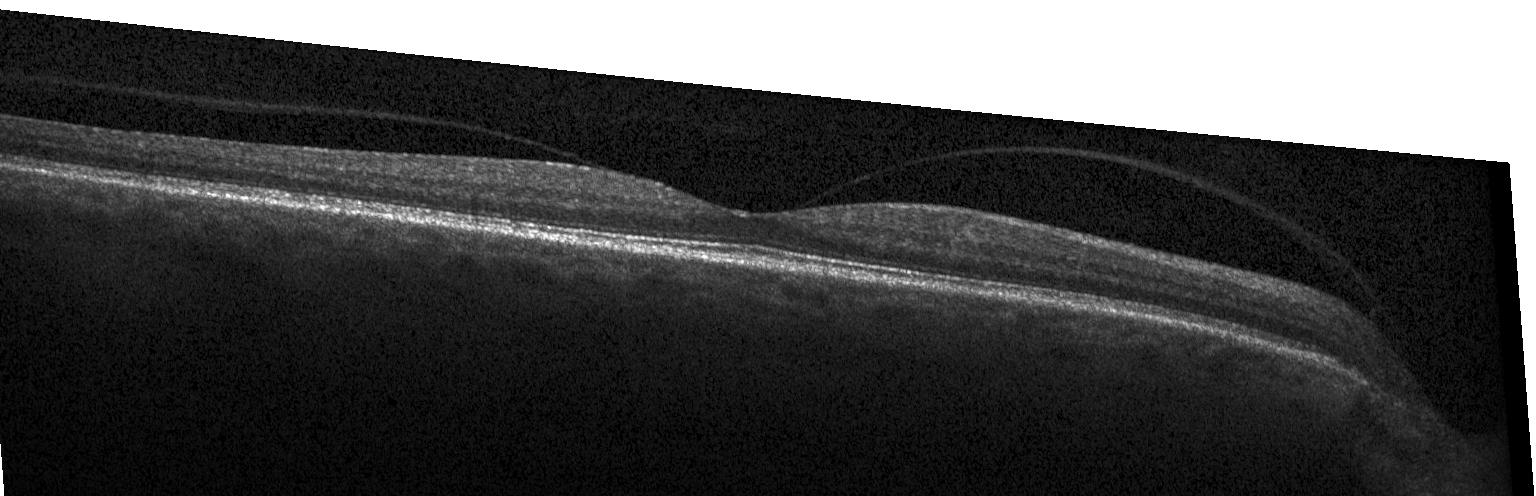
SD-OCT. Optical coherence tomography scan — Finding: neither CNV, DME, nor drusen.